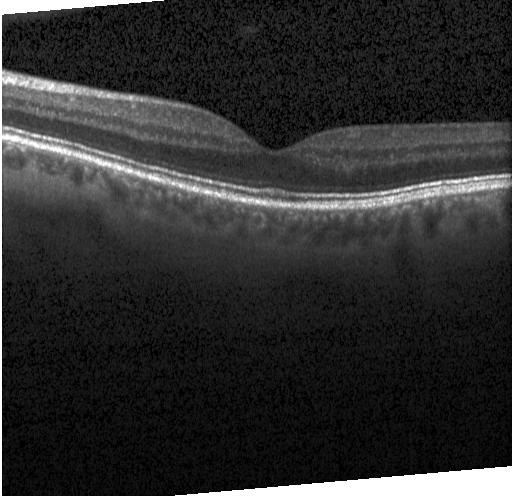

OCT scan showing neither CNV, DME, nor drusen.